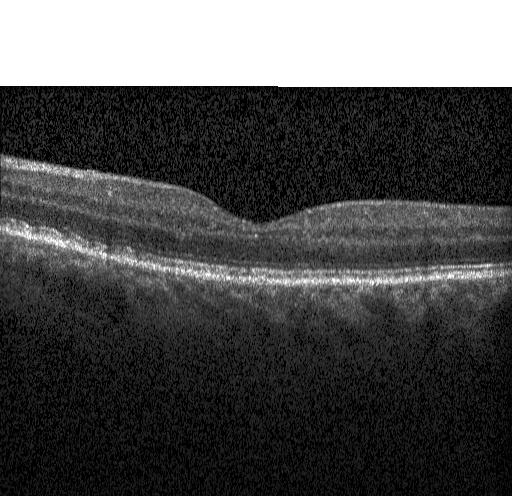
Diagnosis: multiple drusen.